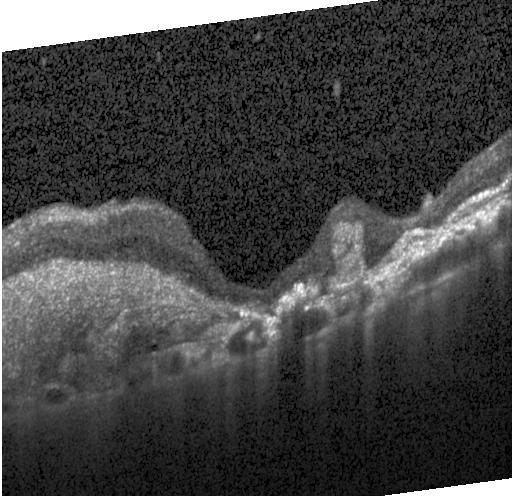

OCT finding: a choroidal neovascular membrane.